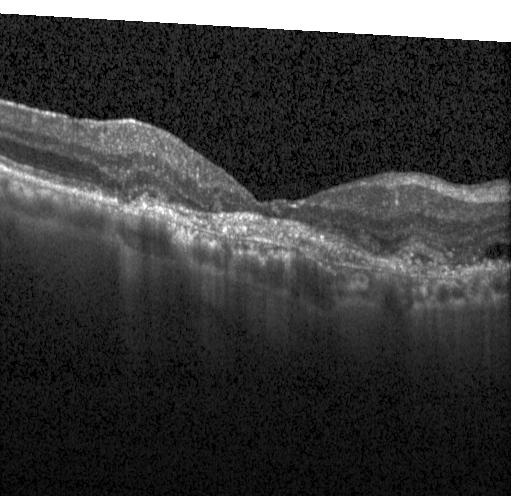 Macular OCT demonstrating a choroidal neovascular membrane.